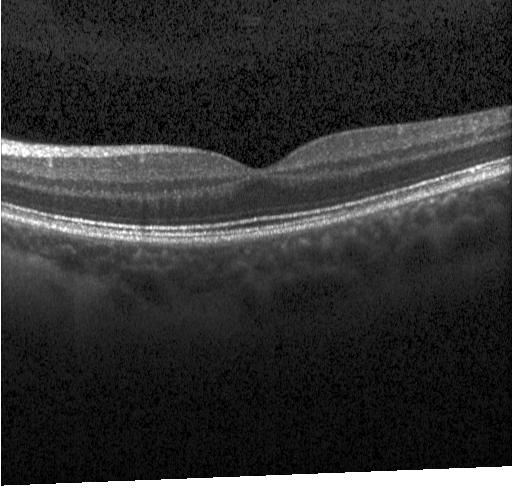

OCT B-scan
Diagnosis: neither choroidal neovascularization, diabetic macular edema, nor drusen.